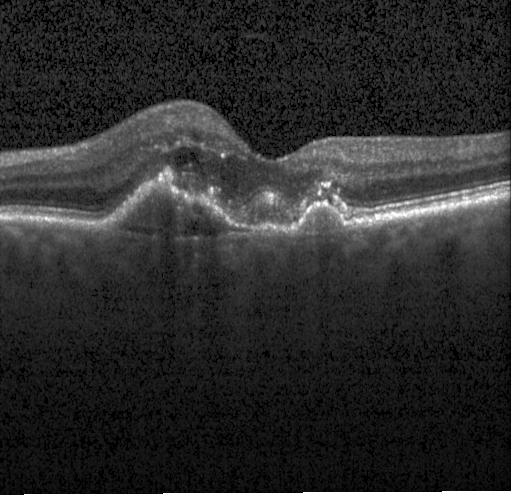
OCT scan showing a choroidal neovascular membrane.